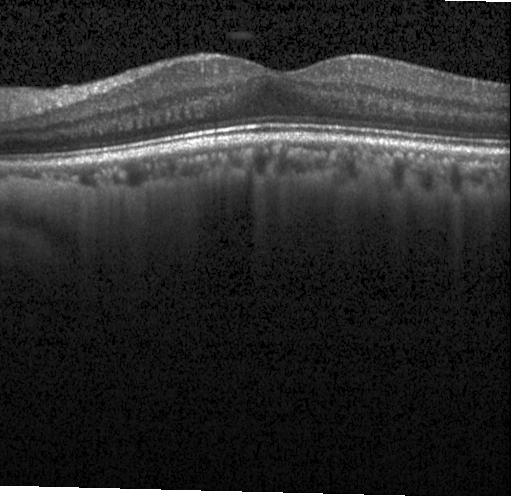
Retinal OCT cross-section showing no choroidal neovascularization, diabetic macular edema, or drusen.